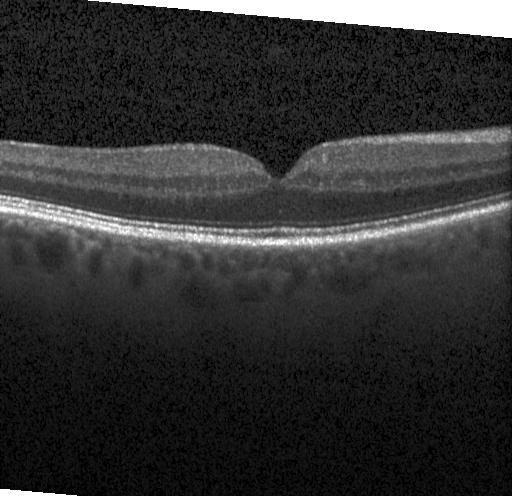 Neither choroidal neovascularization, diabetic macular edema, nor drusen.